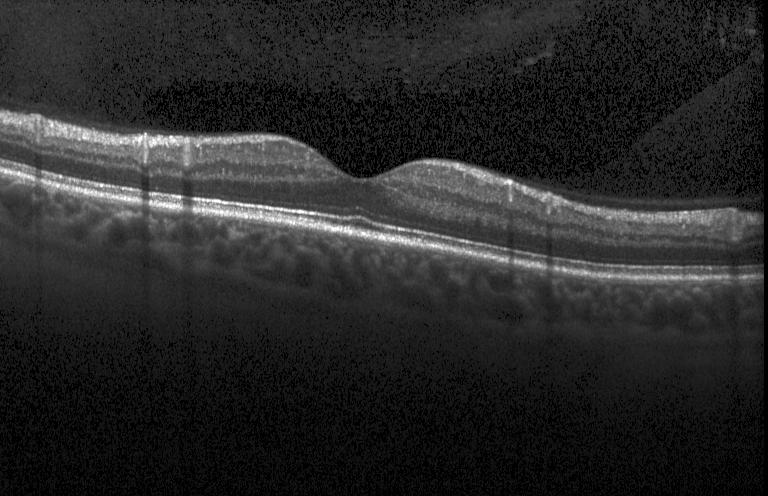
Assessment: no choroidal neovascularization, diabetic macular edema, or drusen.